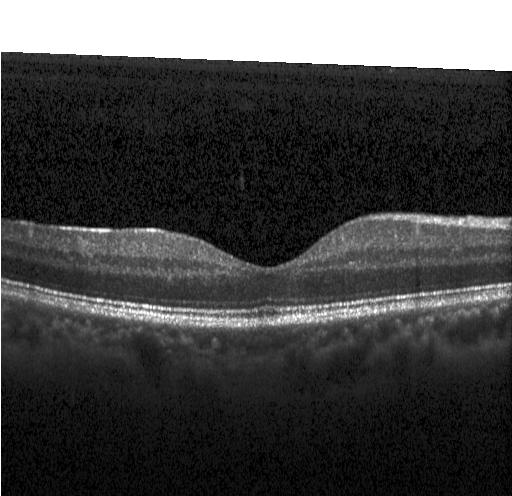
Spectral-domain OCT. Retinal OCT B-scan
No choroidal neovascularization, diabetic macular edema, or drusen.